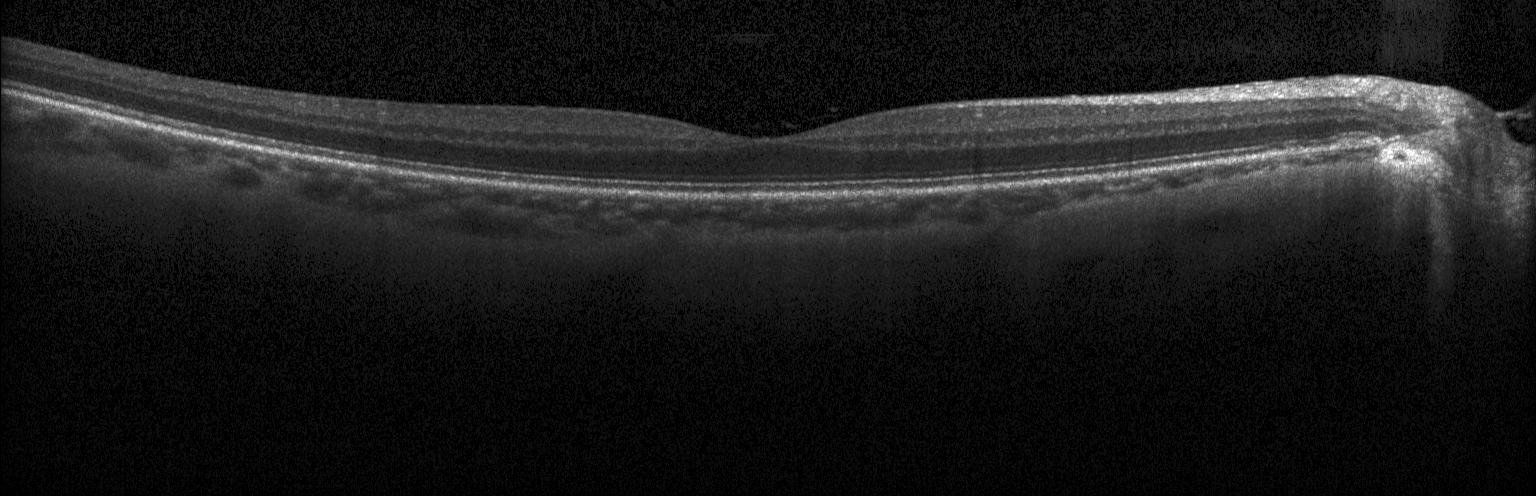 Centered on the fovea, OCT line scan.
Impression: no evidence of CNV, DME, or drusen.